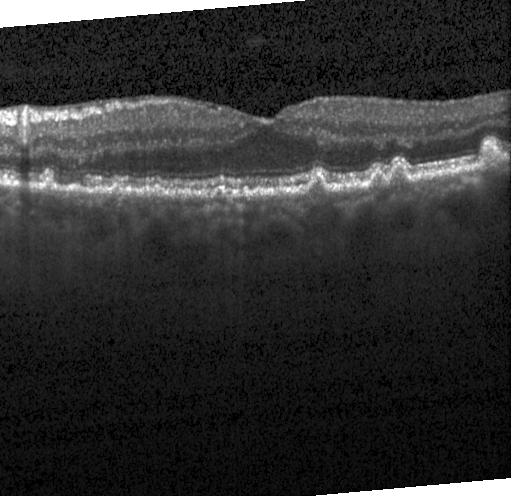
Macular OCT demonstrating multiple drusen.